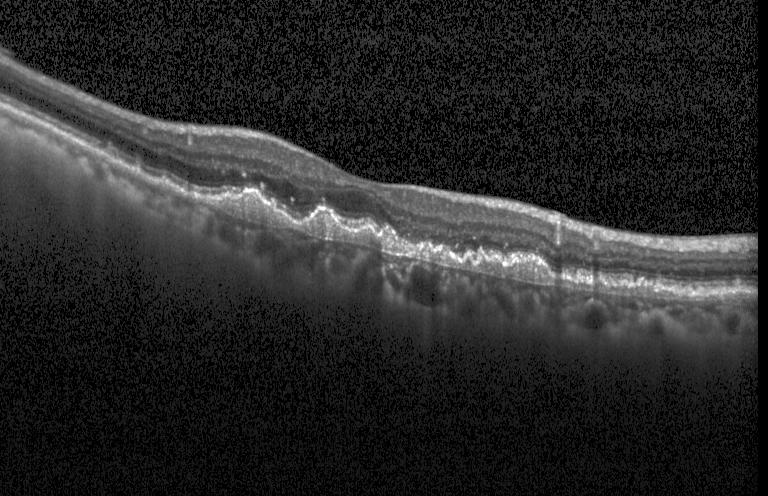 Assessment: choroidal neovascularization.